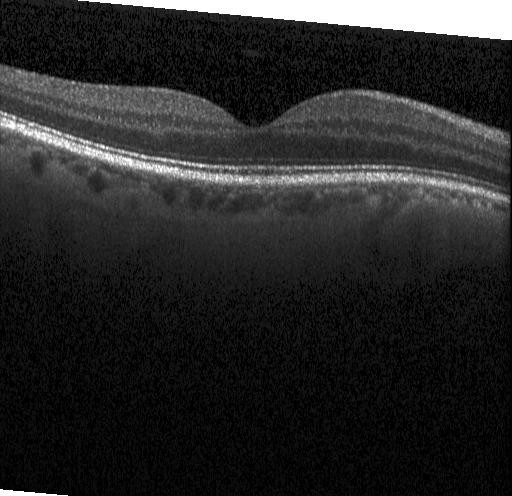 Optical coherence tomography B-scan. Dx: no choroidal neovascularization, diabetic macular edema, or drusen.